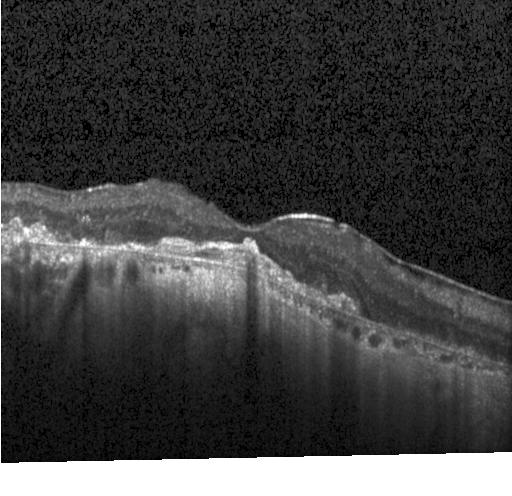

Impression: CNV.